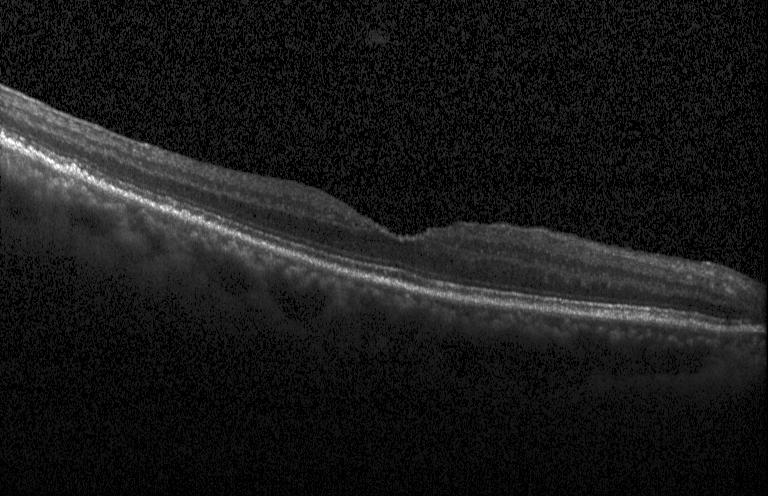 Optical coherence tomography B-scan. No evidence of choroidal neovascularization, diabetic macular edema, or drusen.